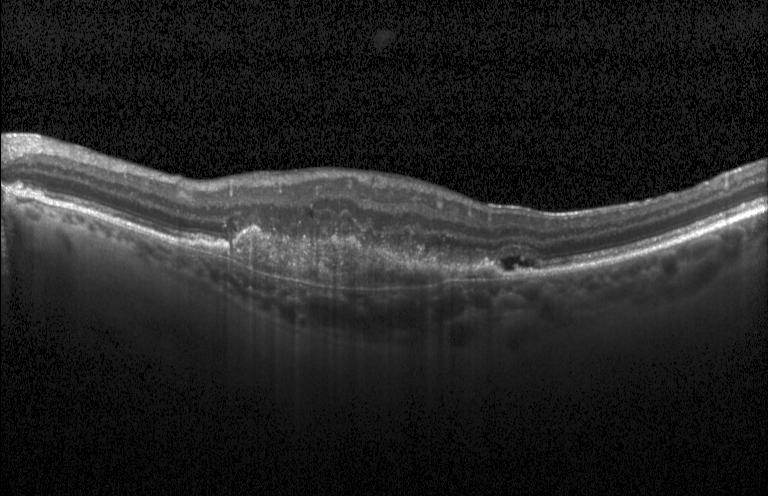

Retinal OCT B-scan. Horizontal scan through the fovea. Instrument: Heidelberg Spectralis. SD-OCT.
Diagnosis: a choroidal neovascular membrane.